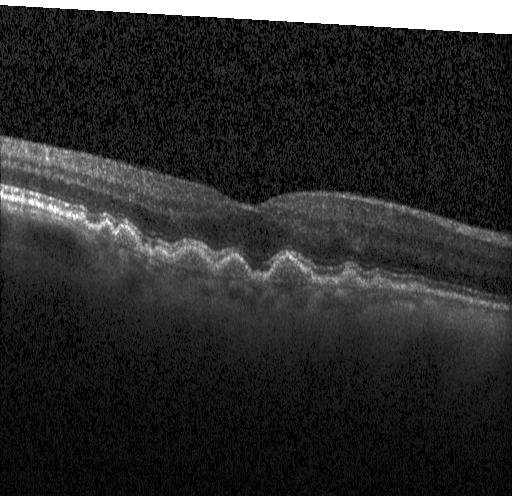

OCT B-scan. Dx: sub-RPE drusenoid deposits.